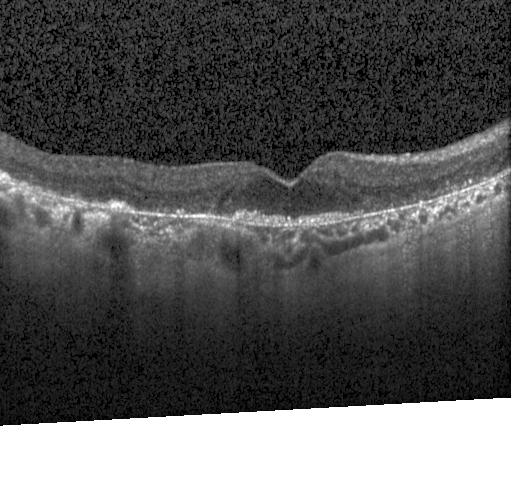 Dx: a choroidal neovascular membrane.